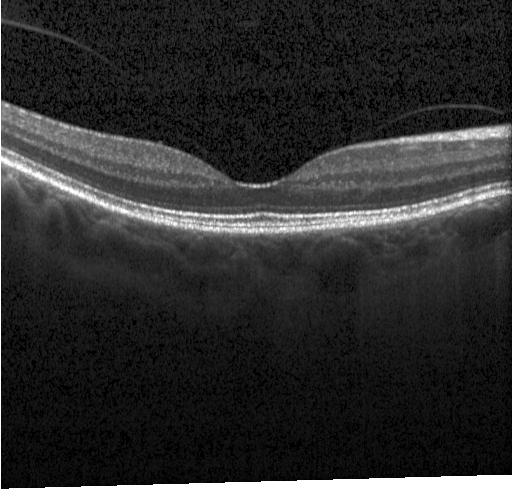

OCT line scan. OCT finding: neither choroidal neovascularization, diabetic macular edema, nor drusen.